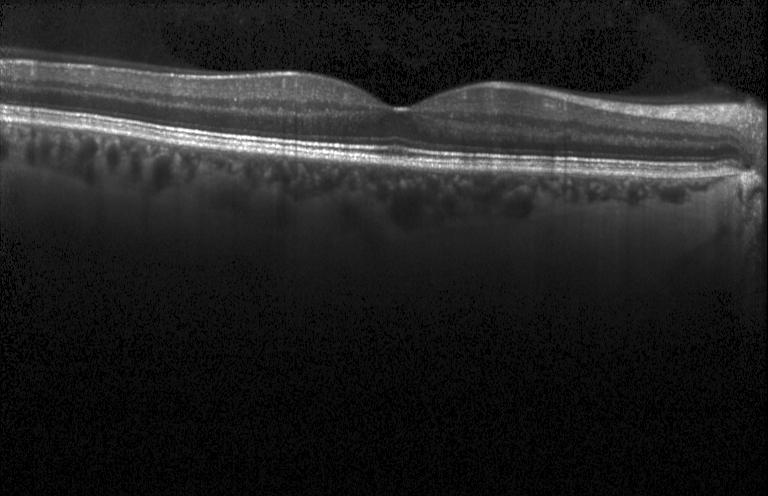

Diagnosis: no choroidal neovascularization, no diabetic macular edema, and no drusen.